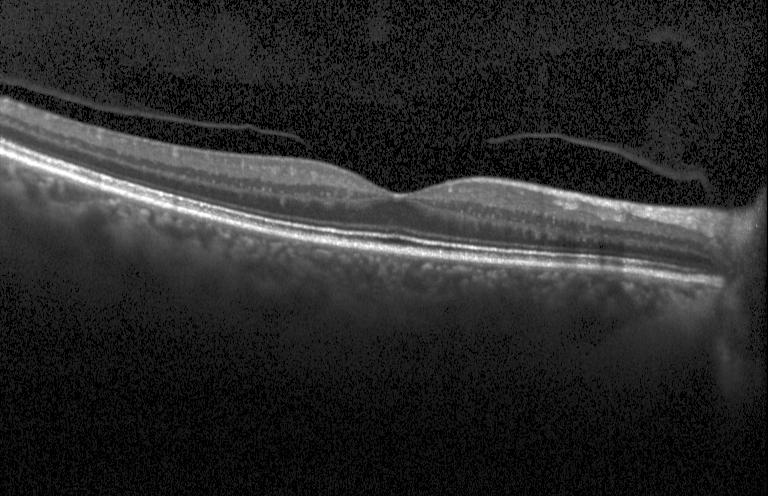
Heidelberg Spectralis OCT system, horizontal scan through the fovea, spectral-domain OCT, retinal OCT B-scan.
No evidence of choroidal neovascularization, diabetic macular edema, or drusen.